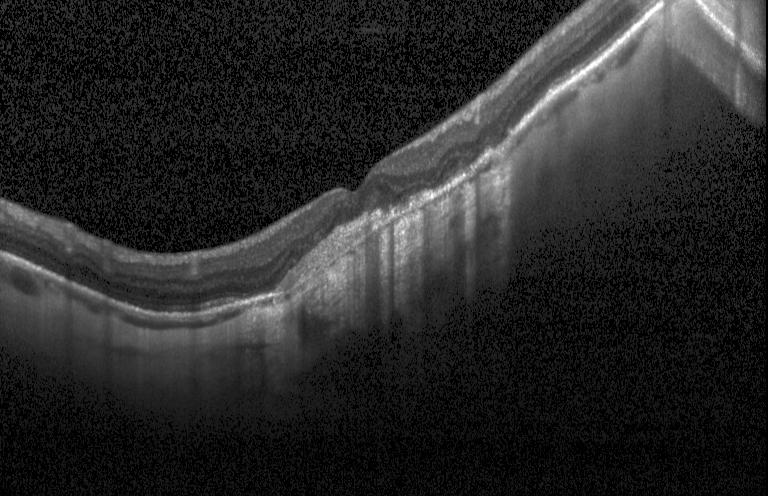

Impression: a choroidal neovascular membrane.